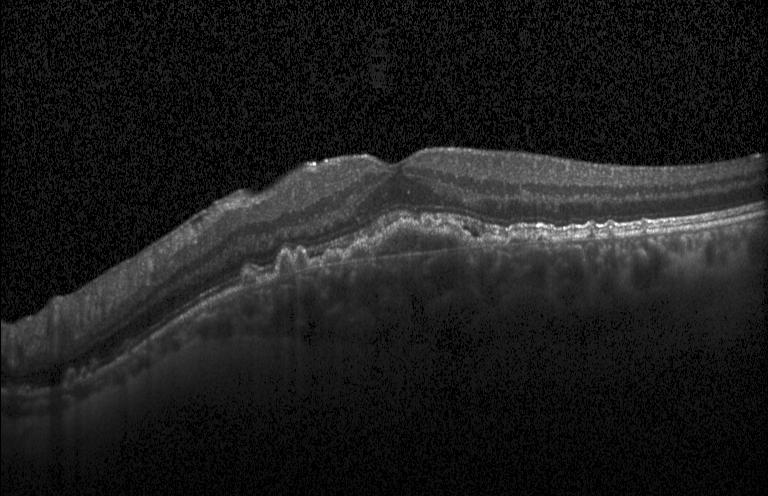 Choroidal neovascularization.